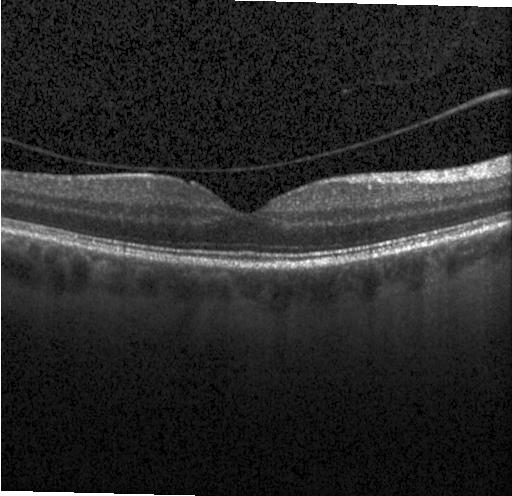

Spectral-domain optical coherence tomography. Horizontal scan through the fovea. OCT B-scan — OCT finding: neither choroidal neovascularization, diabetic macular edema, nor drusen.